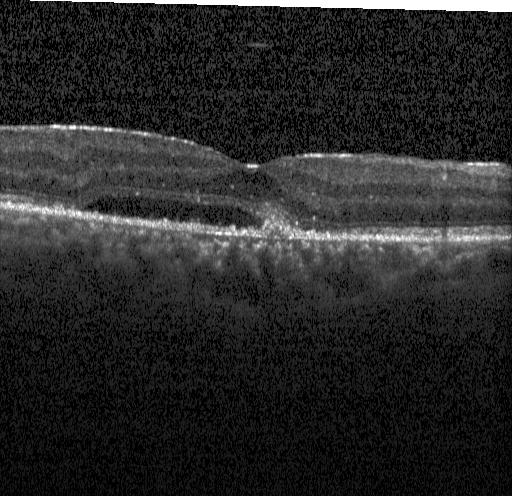 OCT B-scan. SD-OCT. Dx: a choroidal neovascular membrane.